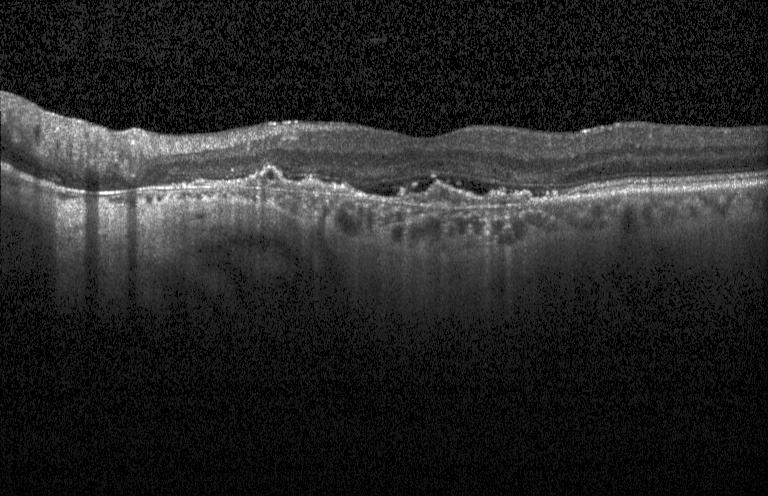

OCT line scan · spectral-domain optical coherence tomography — Diagnosis: a choroidal neovascular membrane.